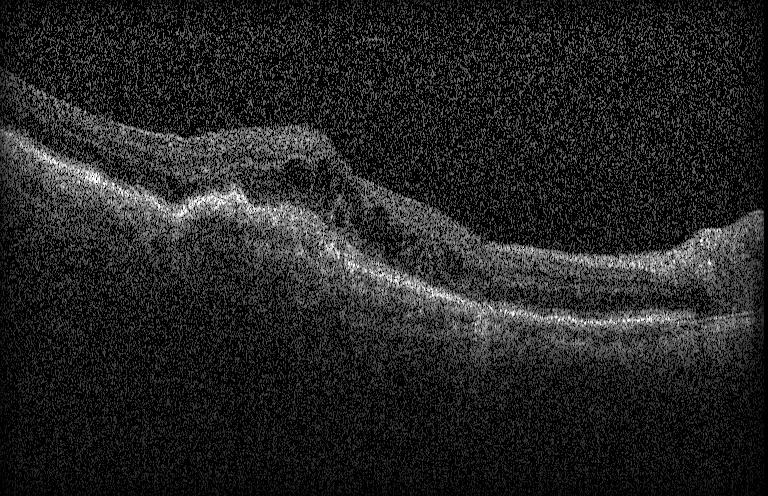

Impression: choroidal neovascularization.